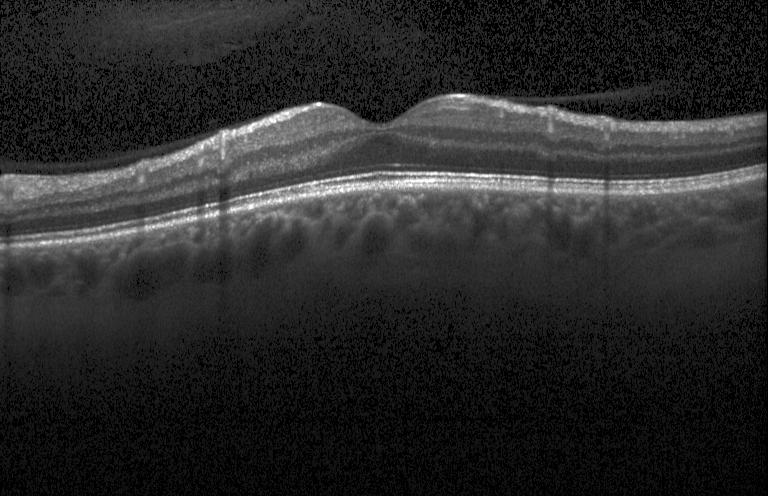
Spectral-domain OCT B-scan: no evidence of choroidal neovascularization, diabetic macular edema, or drusen.